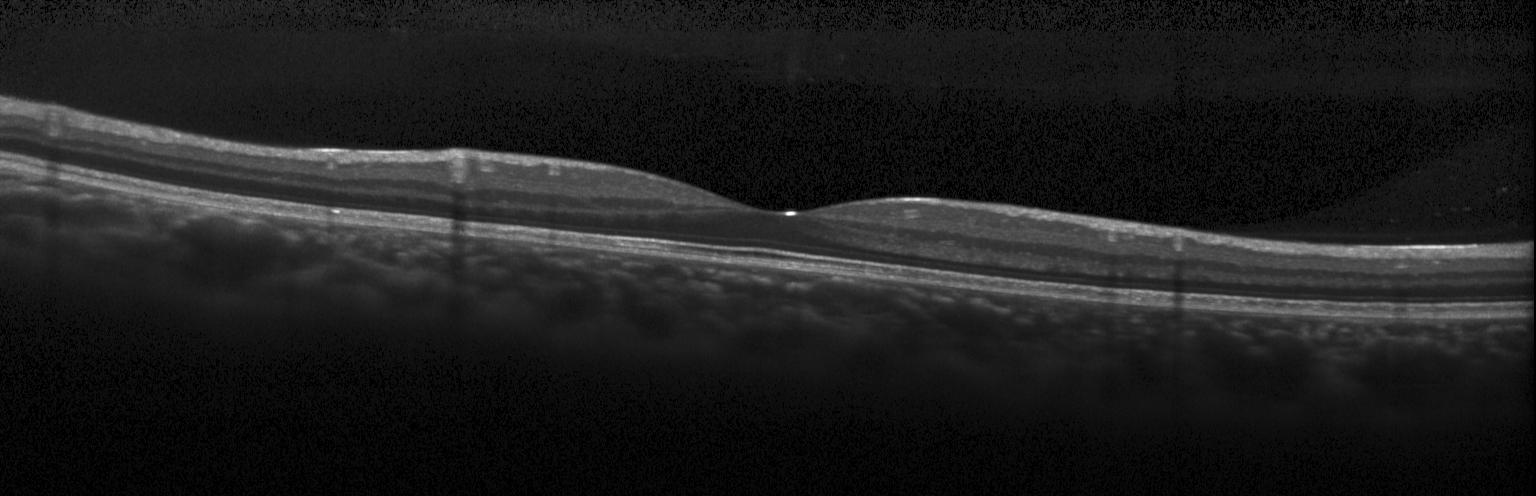 Dx: neither choroidal neovascularization, diabetic macular edema, nor drusen.